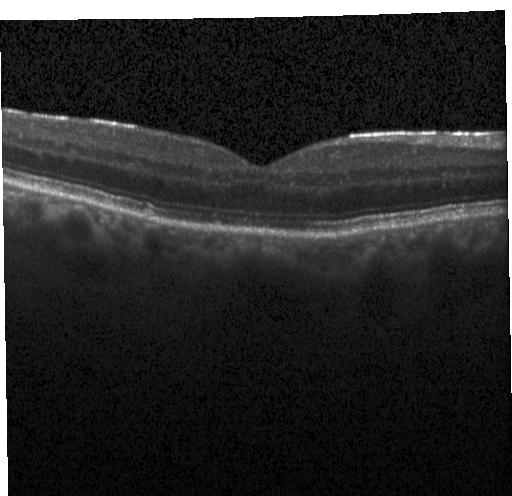
Optical coherence tomography scan · spectral-domain optical coherence tomography · through the macula. Finding: multiple drusen.